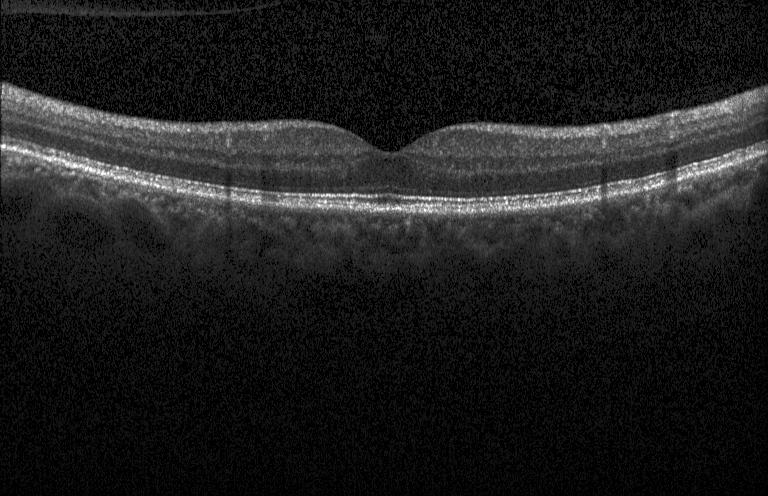 SD-OCT. Retinal OCT cross-section — No choroidal neovascularization, no diabetic macular edema, and no drusen.